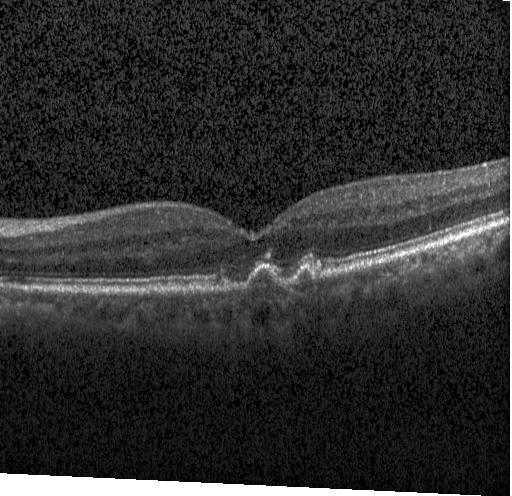

Diagnosis: drusen.